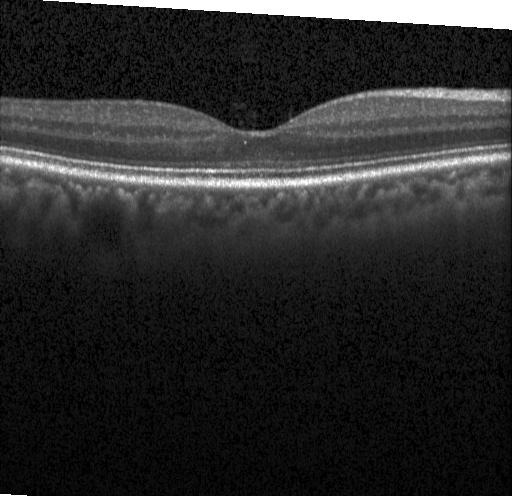

OCT B-scan showing no CNV, no DME, and no drusen.